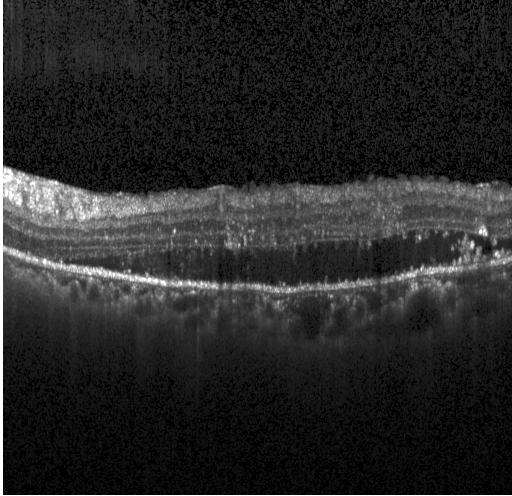 Retinal OCT B-scan. Instrument: Heidelberg Spectralis. Spectral-domain optical coherence tomography. Finding: choroidal neovascularization (CNV).